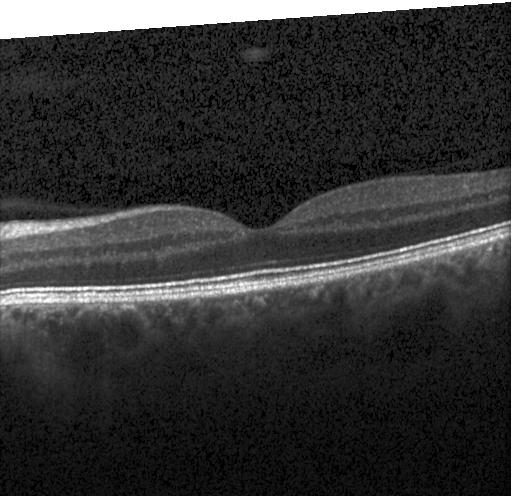 Macular scan; spectral-domain OCT; OCT line scan; instrument: Heidelberg Spectralis. Diagnosis: no choroidal neovascularization, diabetic macular edema, or drusen.